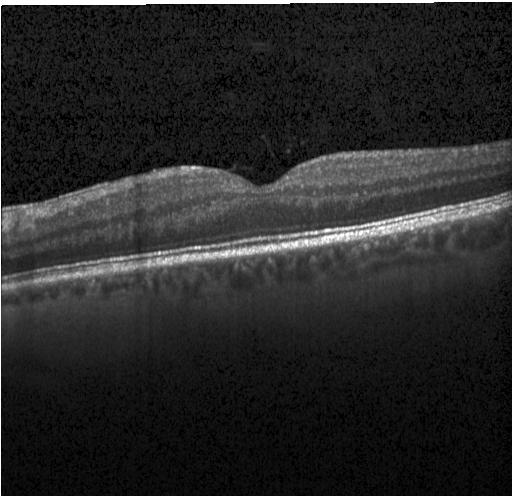 Spectral-domain OCT B-scan: no evidence of choroidal neovascularization, diabetic macular edema, or drusen.